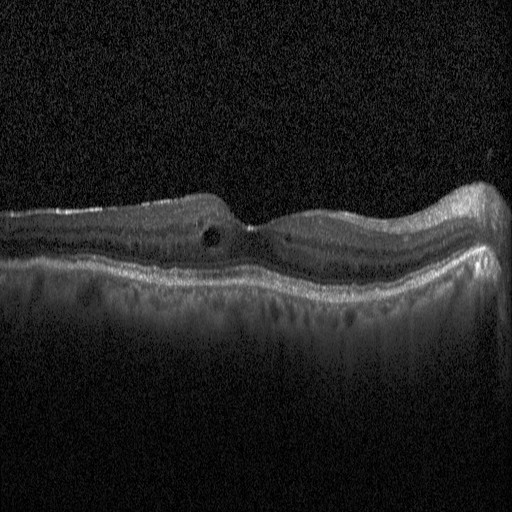
Heidelberg Spectralis OCT system; optical coherence tomography scan; SD-OCT
Impression: diabetic macular edema (DME).